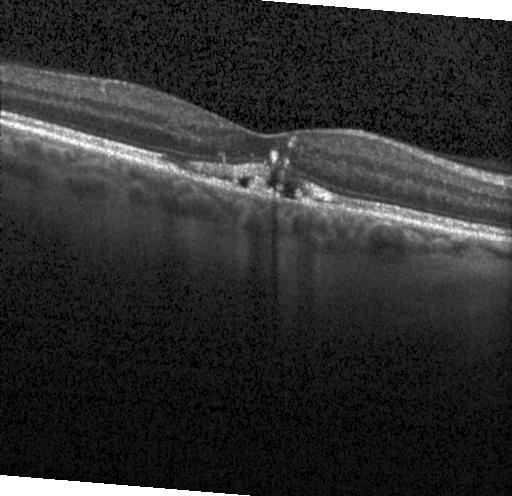
Optical coherence tomography B-scan, instrument: Heidelberg Spectralis.
Diagnosis: CNV.